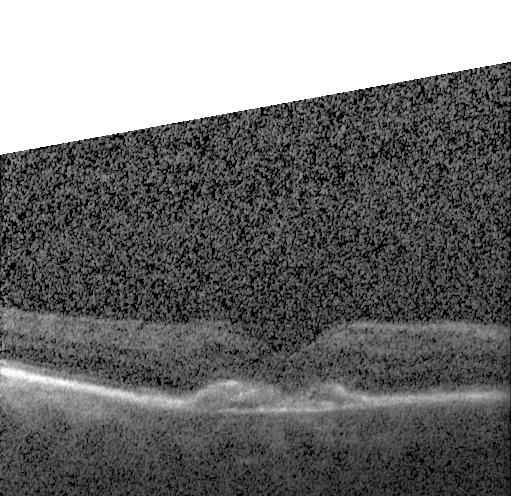
Finding: choroidal neovascularization.